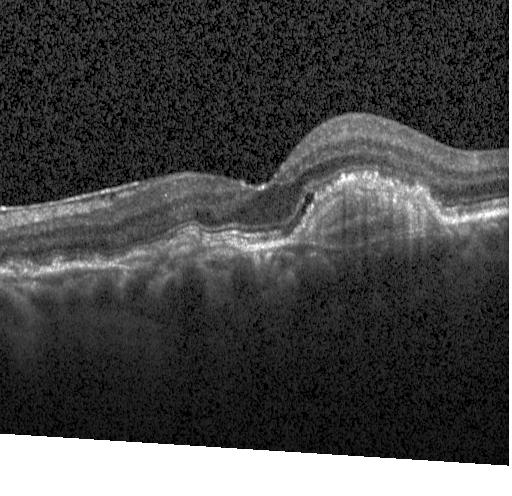
Macular OCT demonstrating a choroidal neovascular membrane.